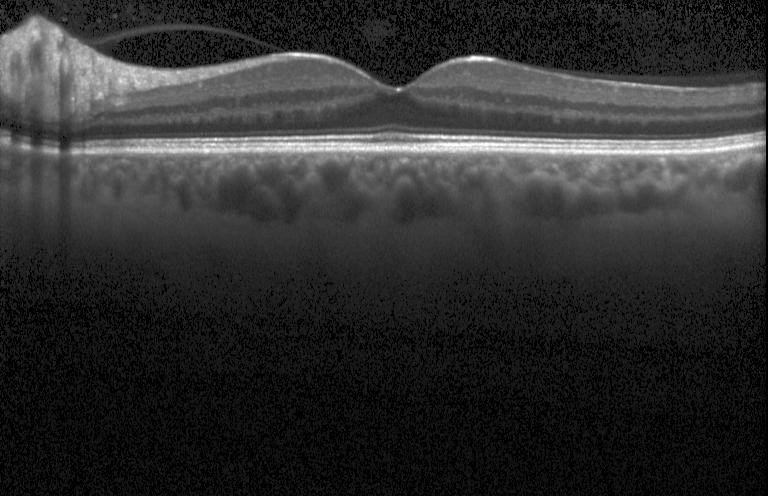 Heidelberg Spectralis · spectral-domain optical coherence tomography · centered on the fovea · retinal OCT B-scan — Impression: no choroidal neovascularization, diabetic macular edema, or drusen.